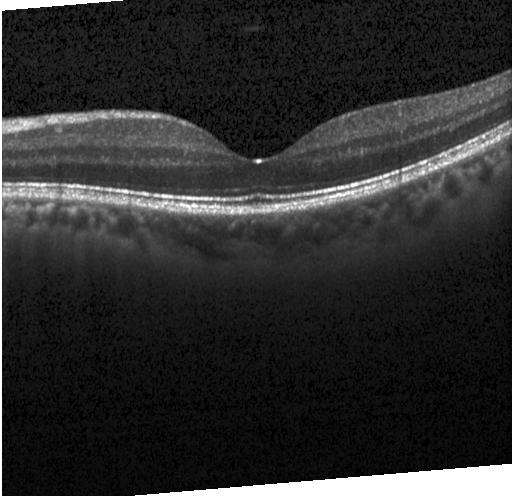 SD-OCT; OCT line scan; centered on the fovea; acquired on a Heidelberg Spectralis. The scan shows neither choroidal neovascularization, diabetic macular edema, nor drusen.